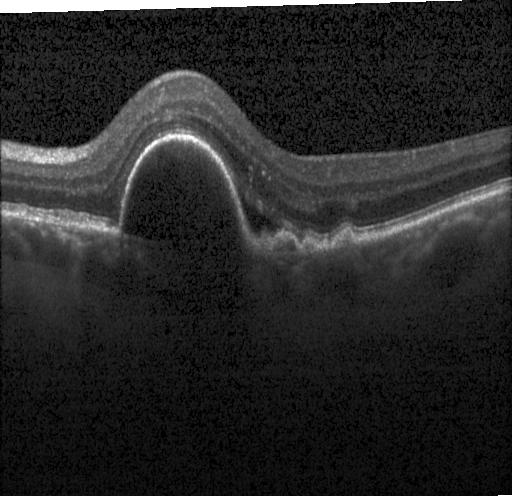
Macular OCT: choroidal neovascularization.